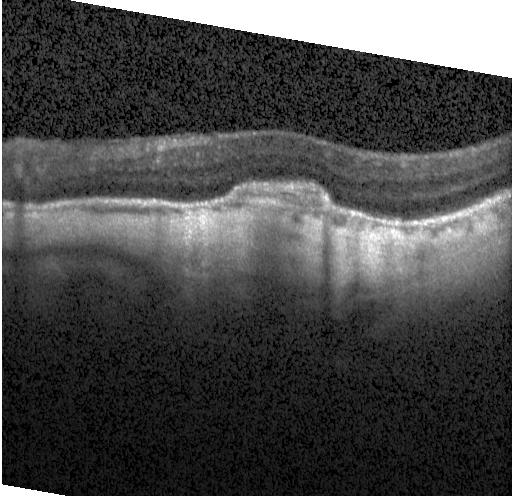

OCT line scan, instrument: Heidelberg Spectralis, fovea-centered — Dx: CNV.